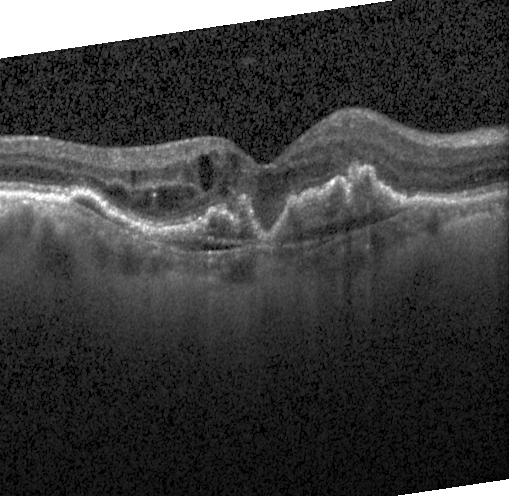 Assessment: choroidal neovascularization.